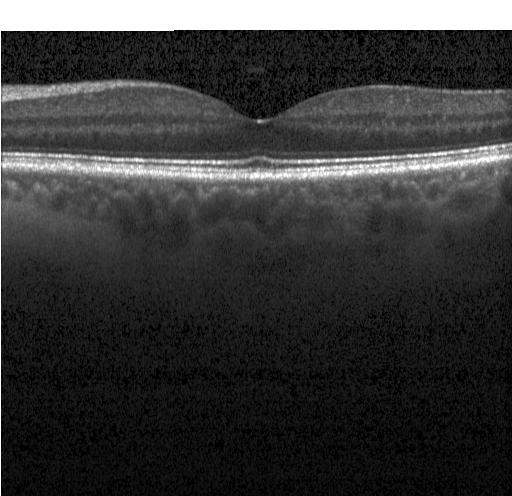
Impression: neither choroidal neovascularization, diabetic macular edema, nor drusen.